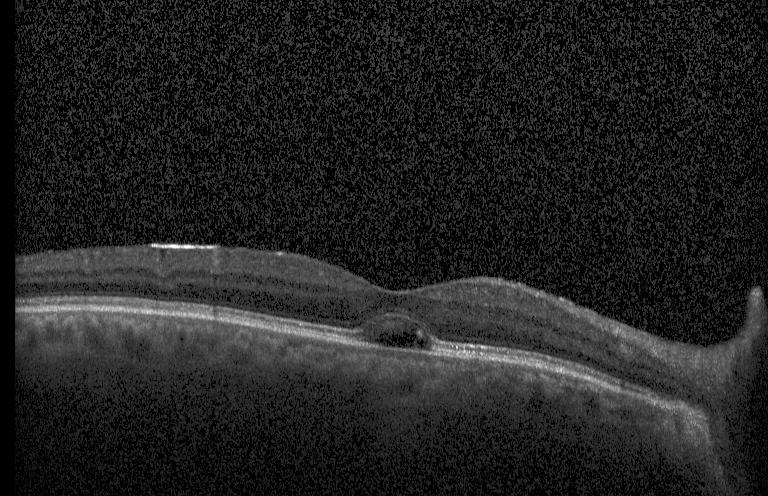 Impression: choroidal neovascularization (CNV).